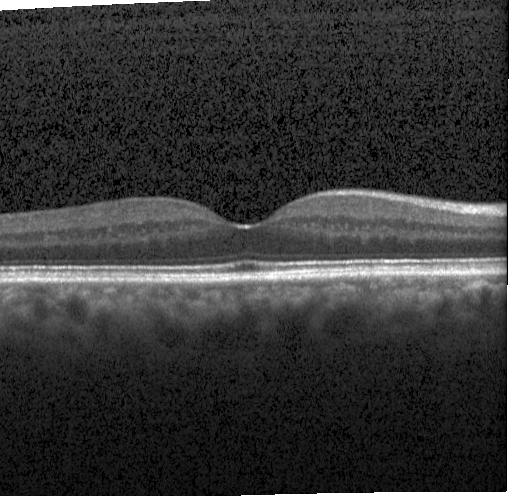 Macular OCT demonstrating neither choroidal neovascularization, diabetic macular edema, nor drusen.